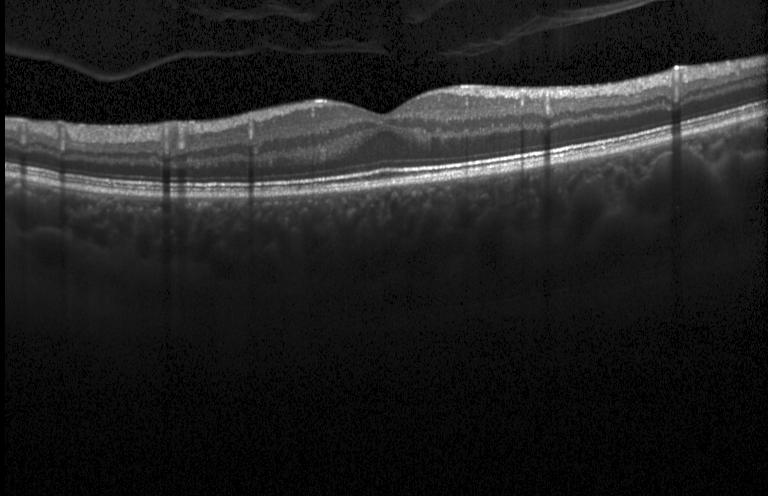 Retinal OCT B-scan · macular scan · SD-OCT · Heidelberg Spectralis OCT system
Impression: no CNV, DME, or drusen.